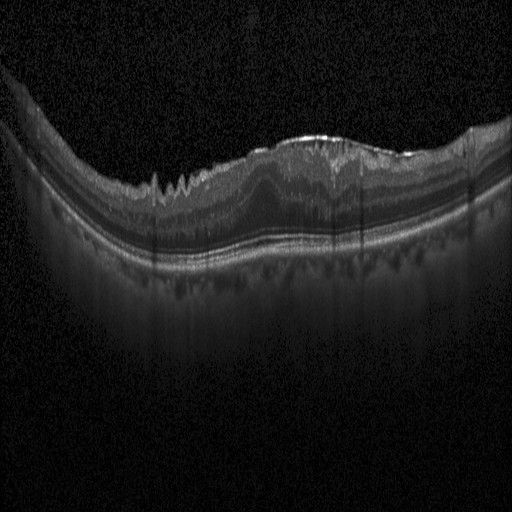 Fovea-centered, instrument: Heidelberg Spectralis, retinal OCT B-scan, spectral-domain OCT. Diagnosis: diabetic macular edema.